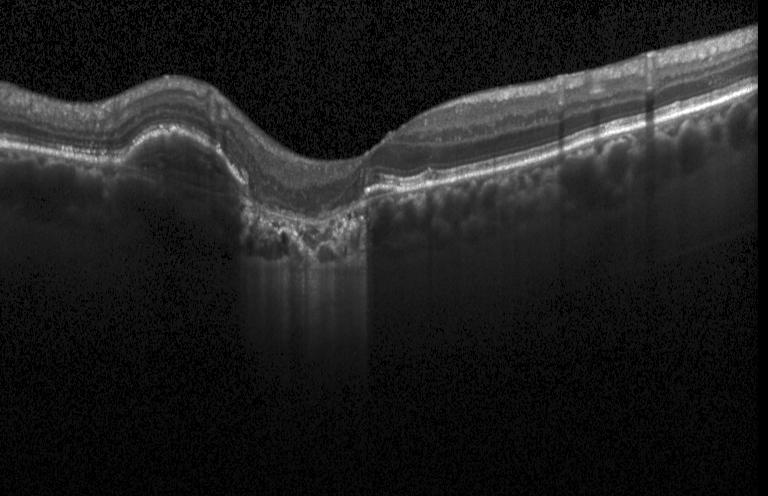

Optical coherence tomography scan, Heidelberg Spectralis OCT system
This B-scan demonstrates a choroidal neovascular membrane.